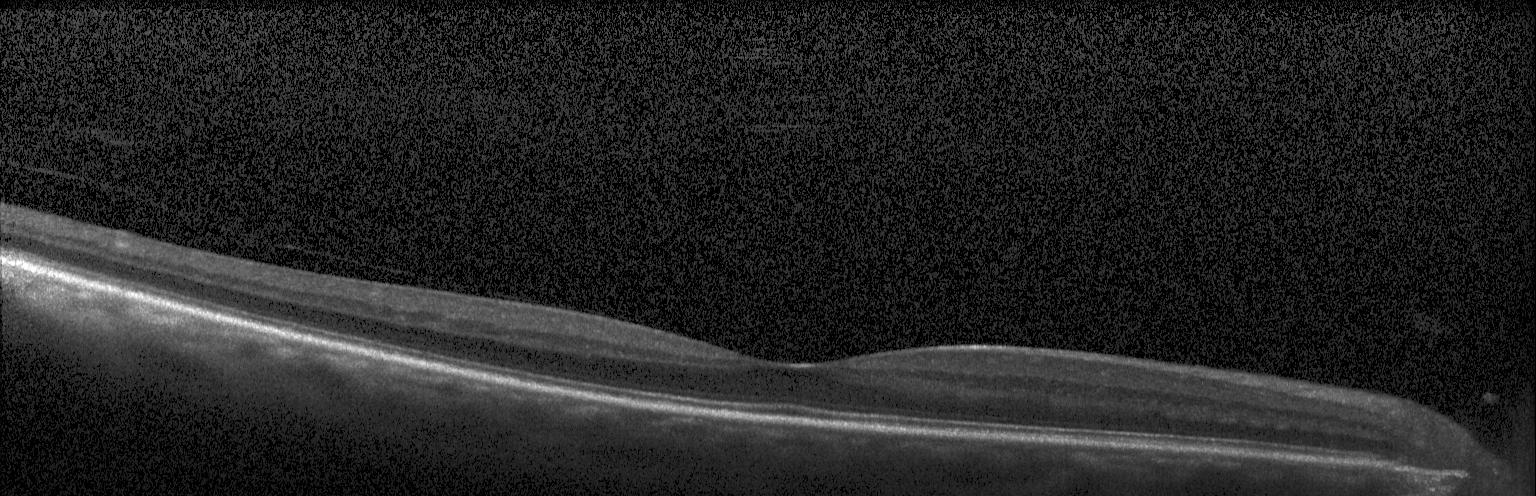

OCT line scan — No choroidal neovascularization, no diabetic macular edema, and no drusen.